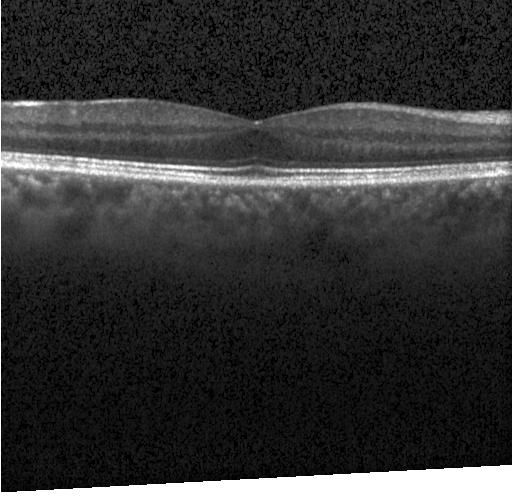
Diagnosis: neither choroidal neovascularization, diabetic macular edema, nor drusen.